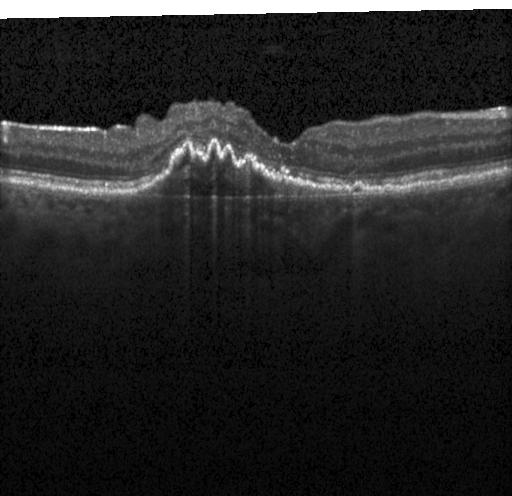
OCT finding: a choroidal neovascular membrane.